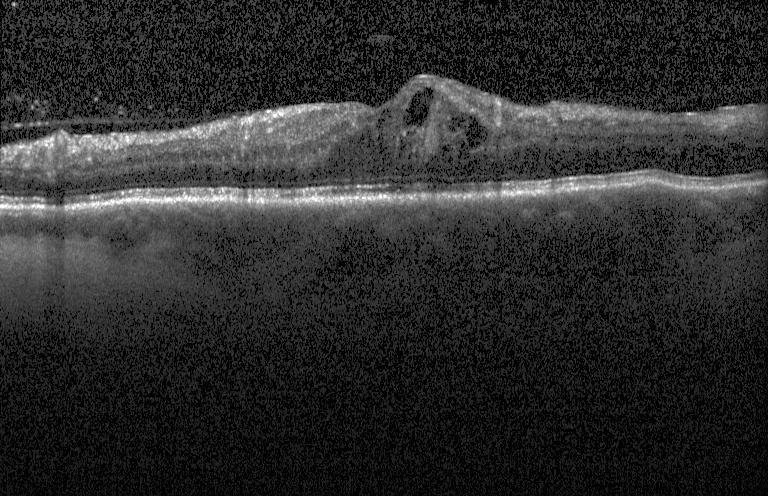
Spectral-domain optical coherence tomography. Through the macula. Heidelberg Spectralis OCT system. Optical coherence tomography scan. Impression: DME.